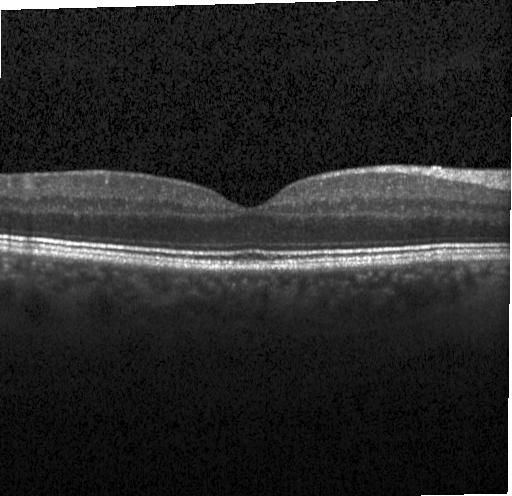
Retinal OCT cross-section
Finding: neither choroidal neovascularization, diabetic macular edema, nor drusen.